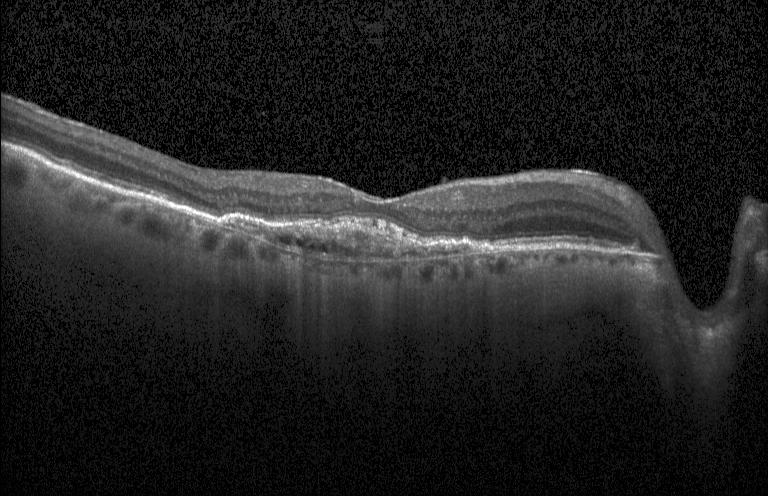 Heidelberg Spectralis OCT system, centered on the fovea, retinal OCT B-scan.
Finding: CNV.